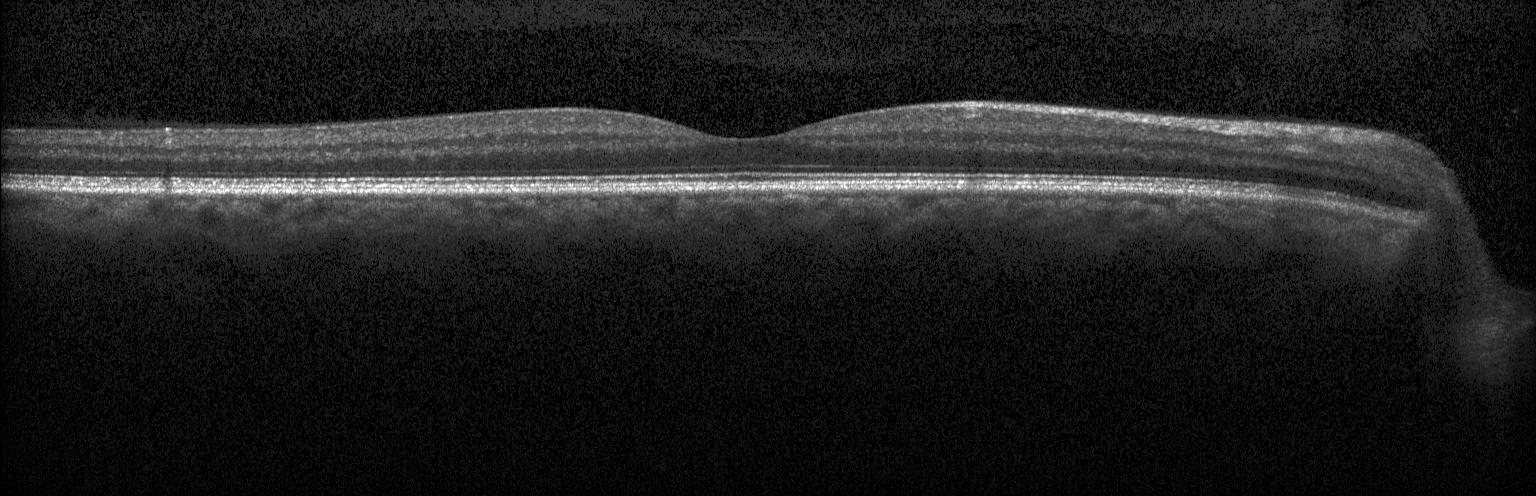 Optical coherence tomography scan; SD-OCT.
The scan shows no choroidal neovascularization, no diabetic macular edema, and no drusen.